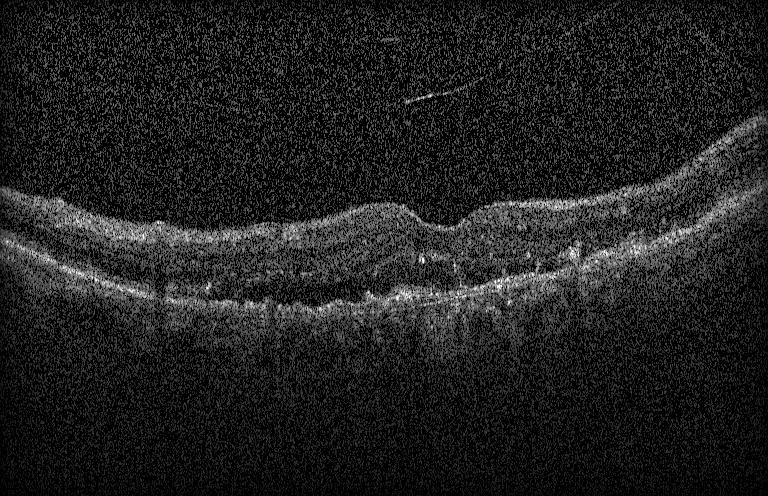
Impression: choroidal neovascularization.